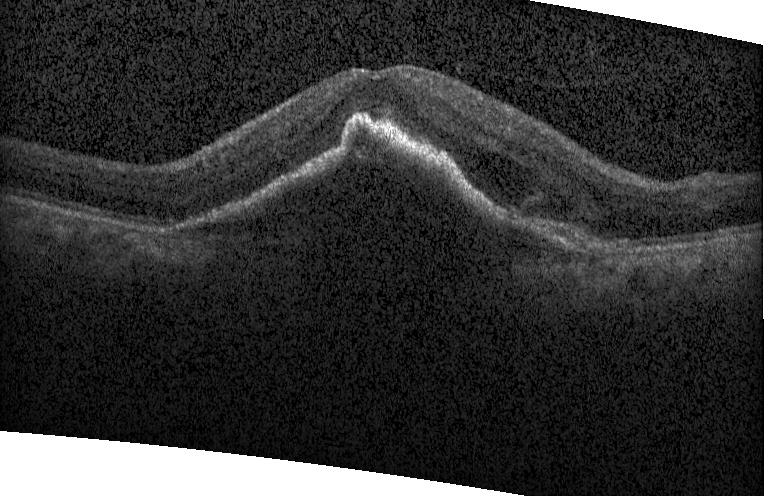

Dx: choroidal neovascularization (CNV).